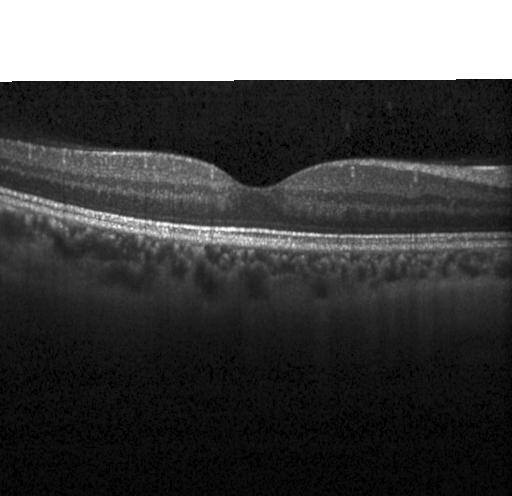

Optical coherence tomography scan · Heidelberg Spectralis OCT system — Diagnosis: no choroidal neovascularization, no diabetic macular edema, and no drusen.